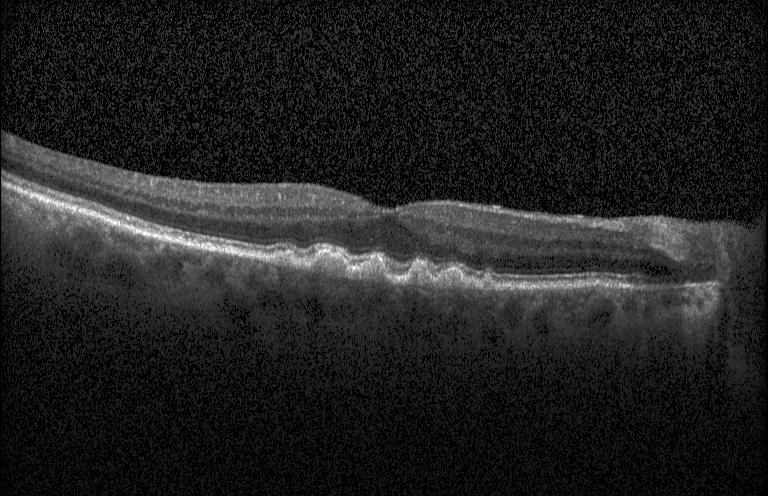 Instrument: Heidelberg Spectralis. Fovea-centered. Retinal OCT cross-section.
This B-scan demonstrates multiple drusen.